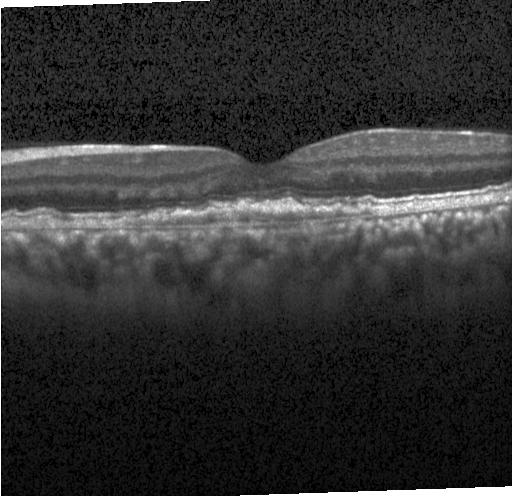 OCT B-scan showing a choroidal neovascular membrane.